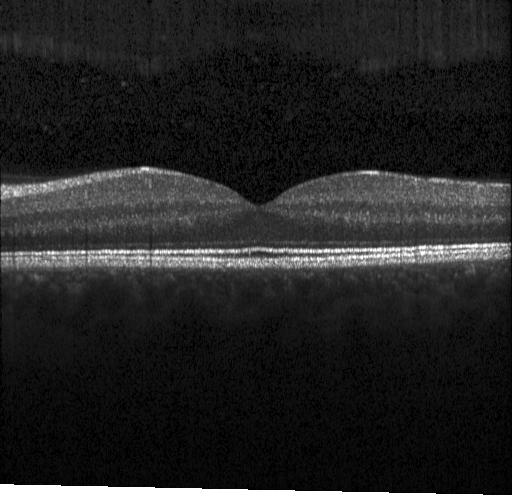 Optical coherence tomography B-scan.
Diagnosis: neither choroidal neovascularization, diabetic macular edema, nor drusen.